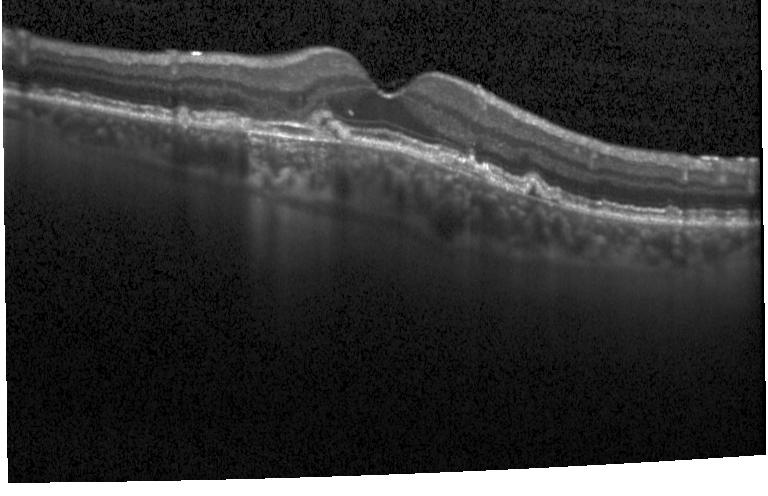

OCT finding: a choroidal neovascular membrane.